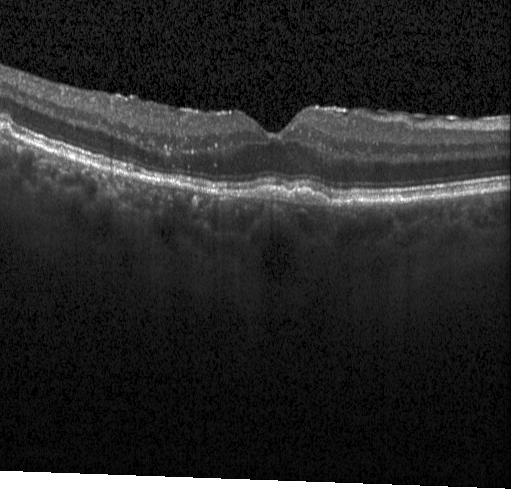 Diagnosis: a choroidal neovascular membrane.